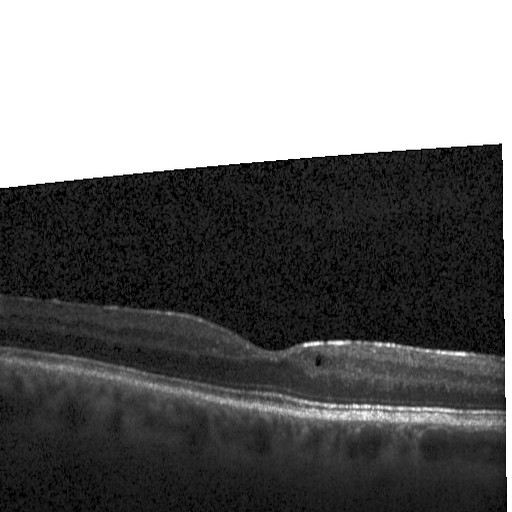

Retinal OCT cross-section; Heidelberg Spectralis OCT system — Impression: DME.